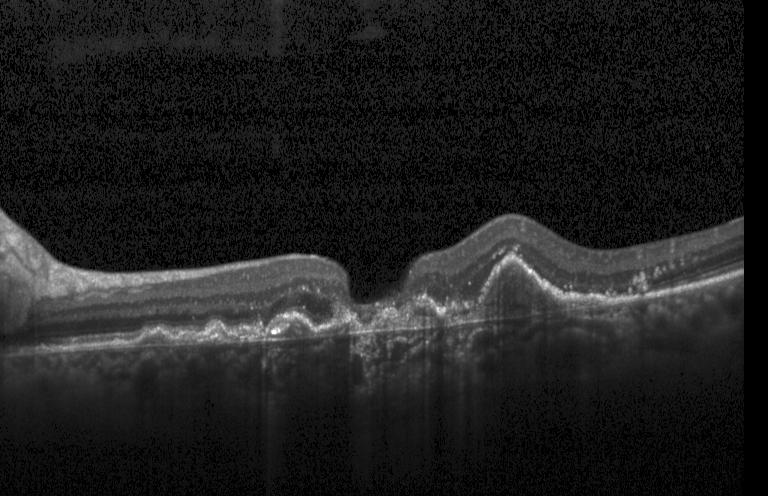

OCT finding: choroidal neovascularization (CNV).